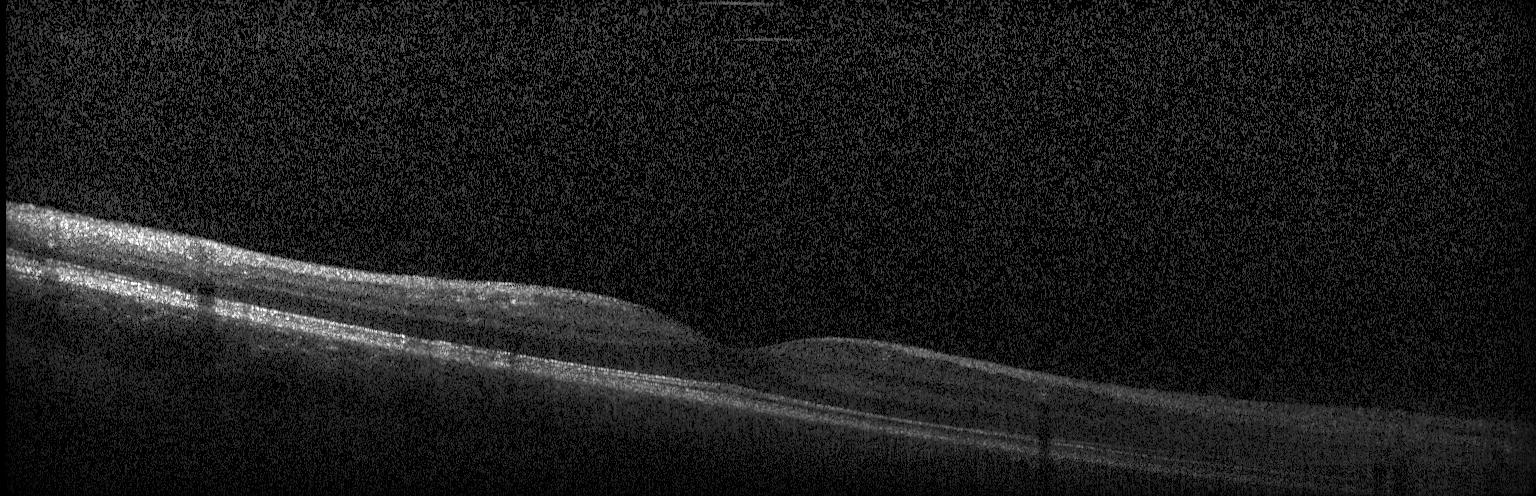 Dx: no evidence of choroidal neovascularization, diabetic macular edema, or drusen.